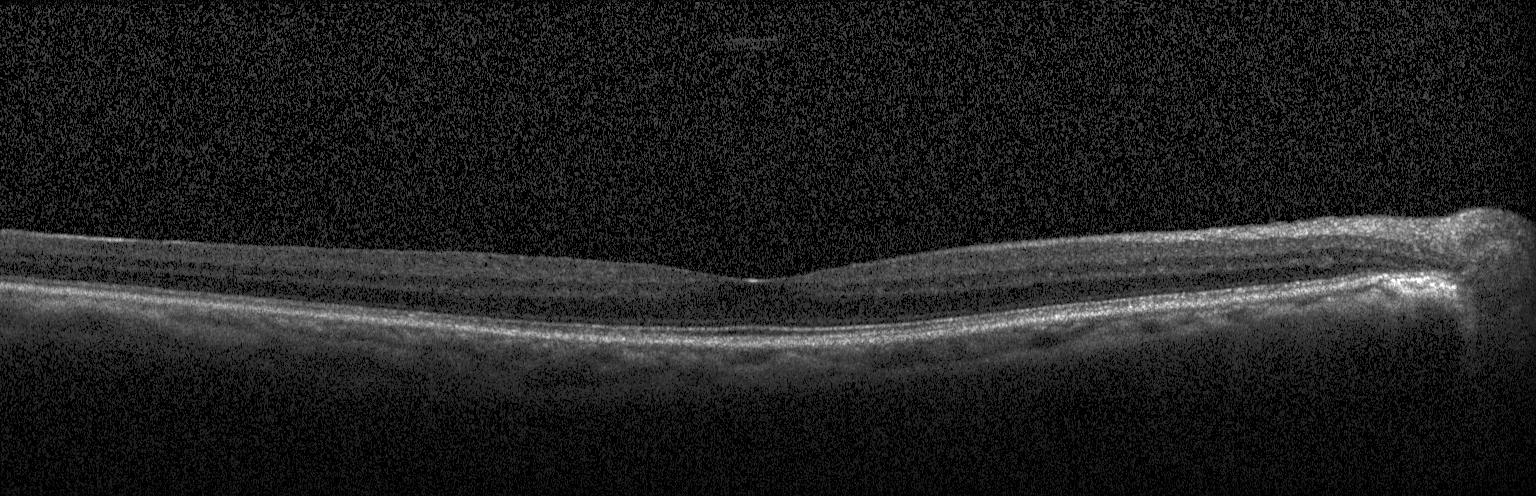 Impression: no choroidal neovascularization, diabetic macular edema, or drusen.